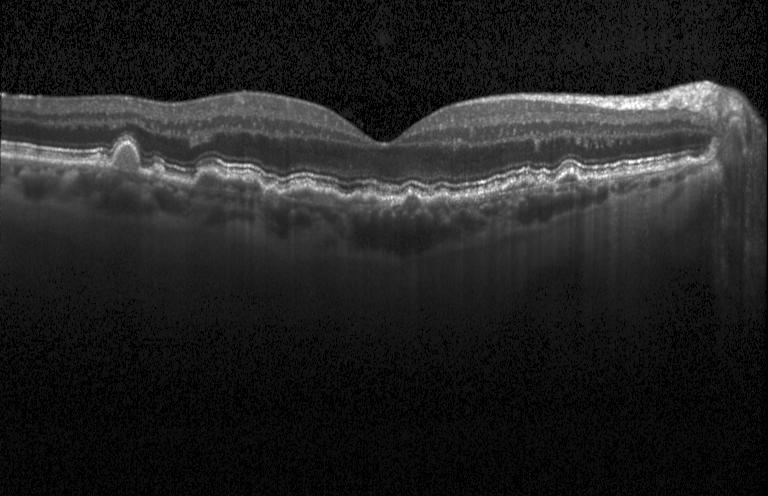 OCT B-scan showing sub-RPE drusenoid deposits.